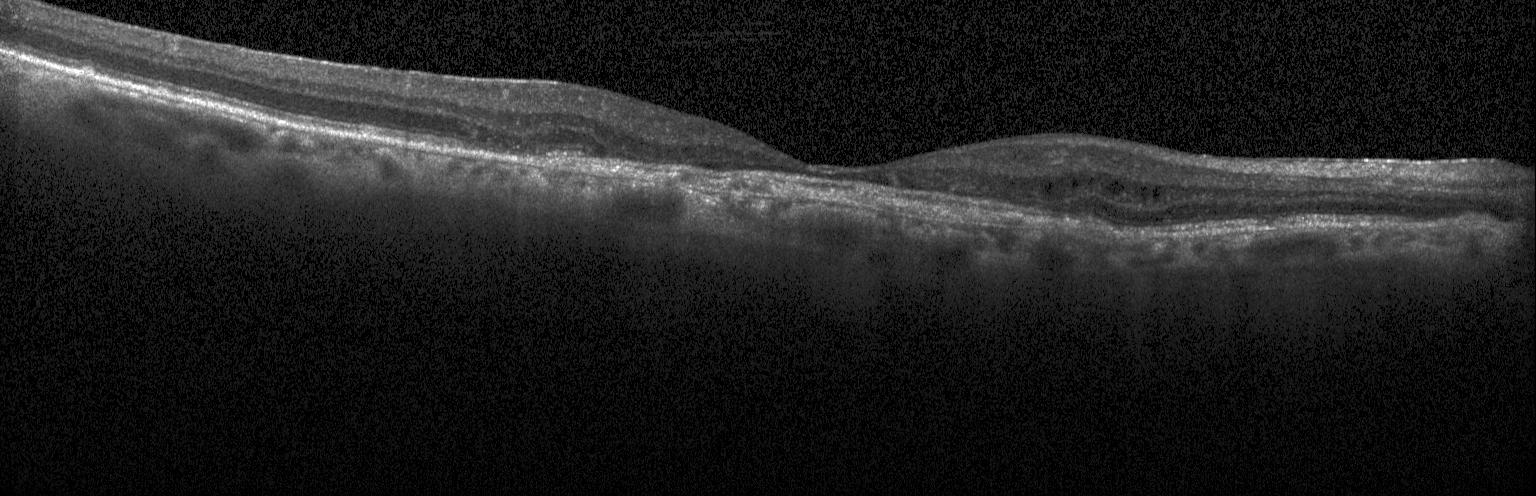 Spectral-domain optical coherence tomography · macular scan · retinal OCT B-scan · Heidelberg Spectralis — Impression: CNV.